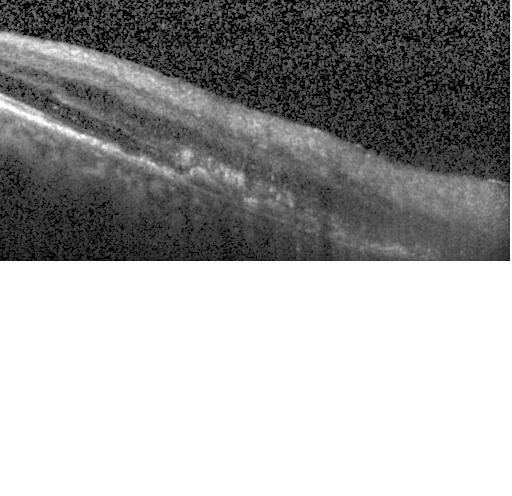 Assessment: choroidal neovascularization.